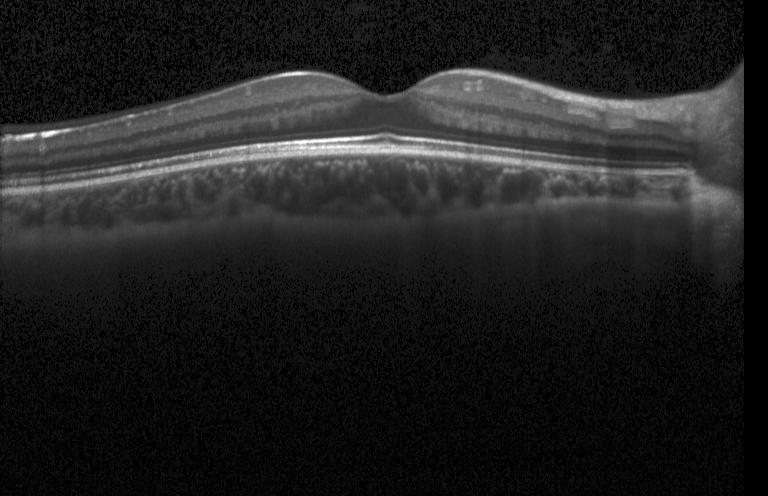 No evidence of CNV, DME, or drusen.